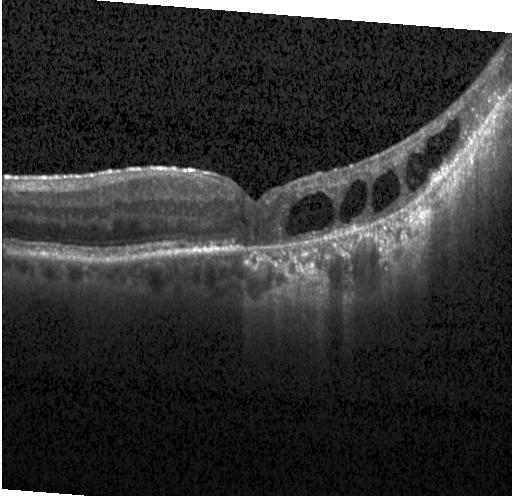
Instrument: Heidelberg Spectralis. Fovea-centered. SD-OCT. OCT line scan — Dx: diabetic macular edema.